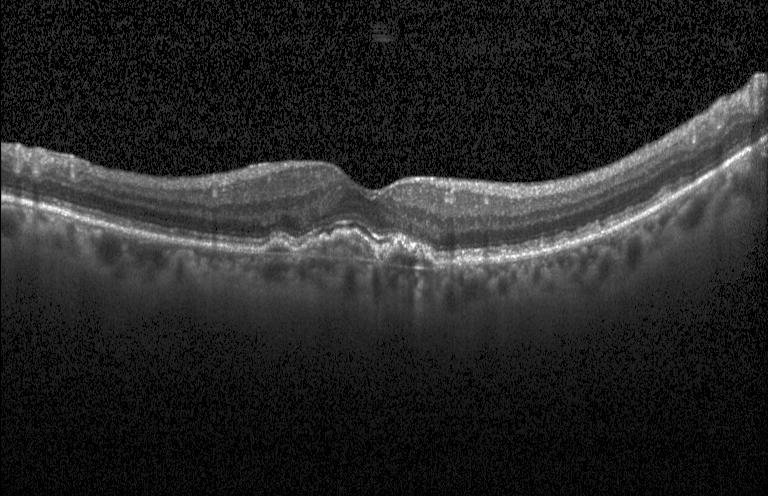

Retinal OCT B-scan. The scan shows CNV.